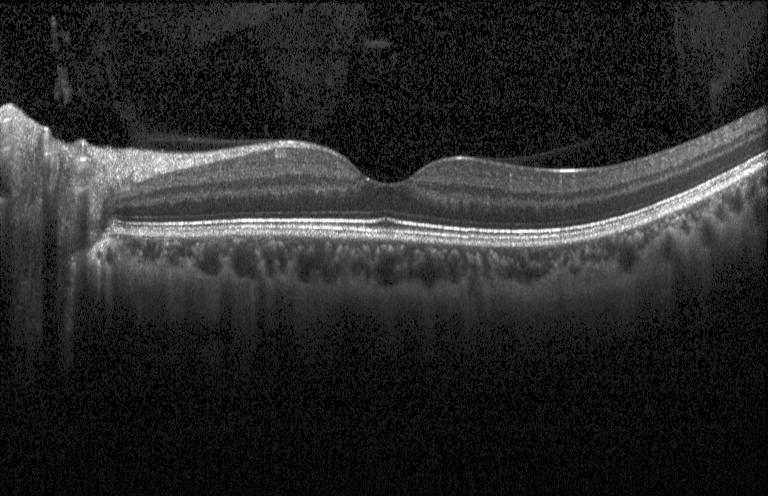
This B-scan demonstrates neither choroidal neovascularization, diabetic macular edema, nor drusen.